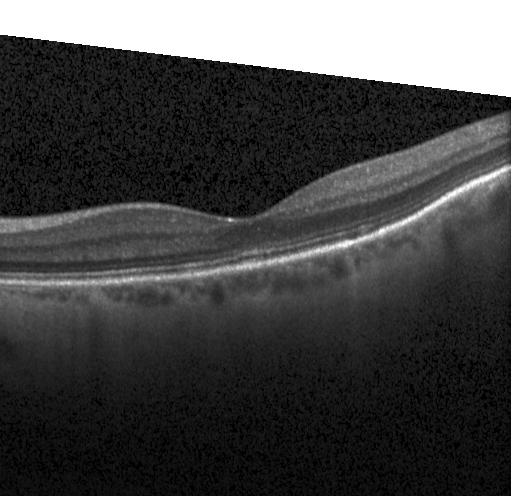
Diagnosis: neither choroidal neovascularization, diabetic macular edema, nor drusen.